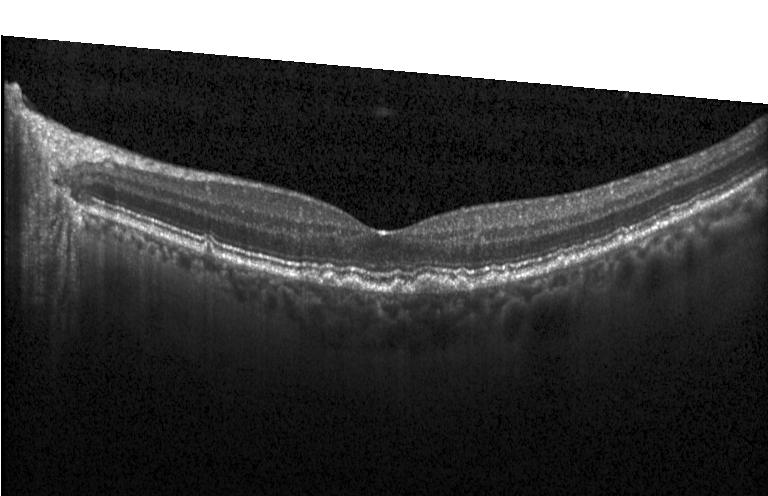
Finding: multiple drusen.